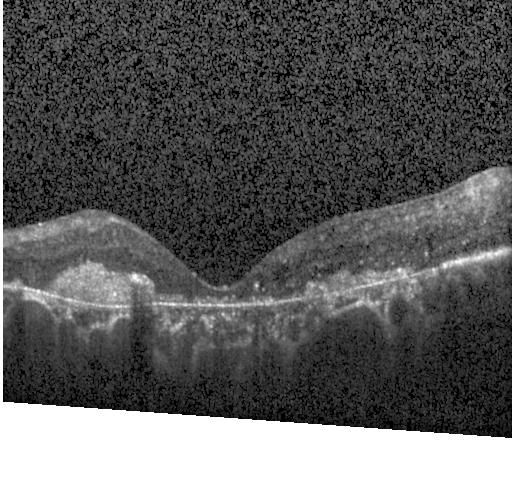
Retinal OCT B-scan. Macular scan.
Impression: a choroidal neovascular membrane.